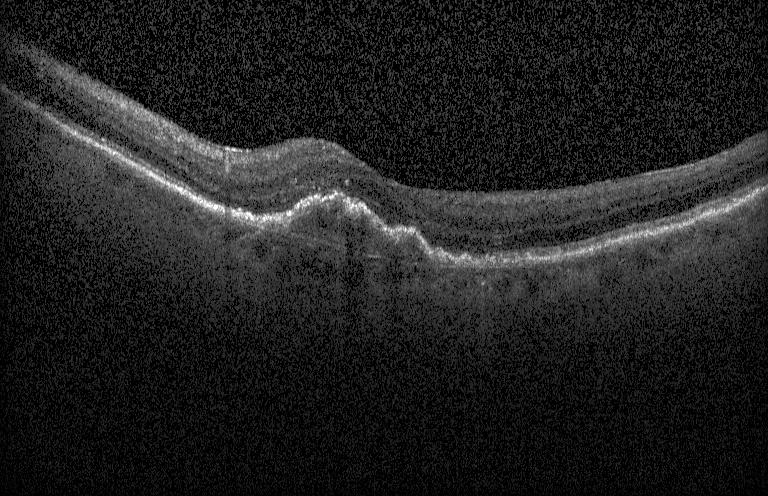

OCT line scan
Assessment: a choroidal neovascular membrane.